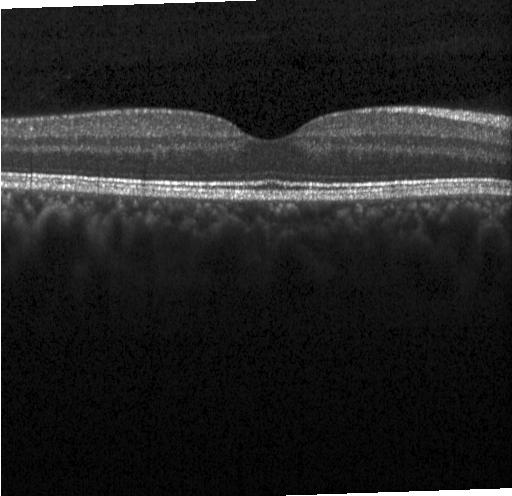

Retinal OCT cross-section, Heidelberg Spectralis, macular scan. Dx: no evidence of choroidal neovascularization, diabetic macular edema, or drusen.